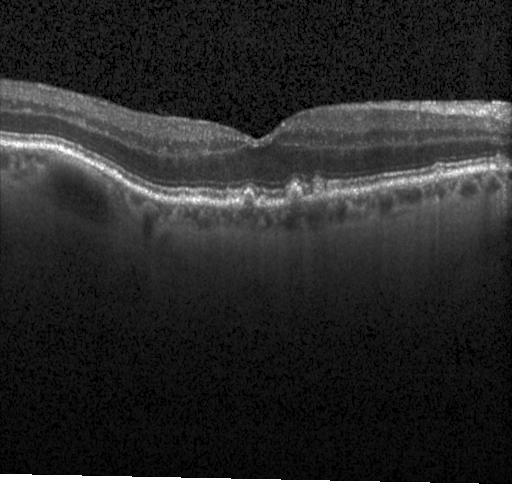 Instrument: Heidelberg Spectralis; optical coherence tomography B-scan; horizontal scan through the fovea; SD-OCT — OCT finding: multiple drusen.